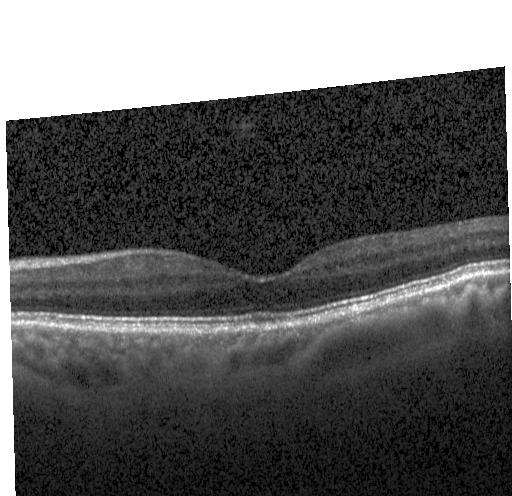
Assessment: no choroidal neovascularization, diabetic macular edema, or drusen.